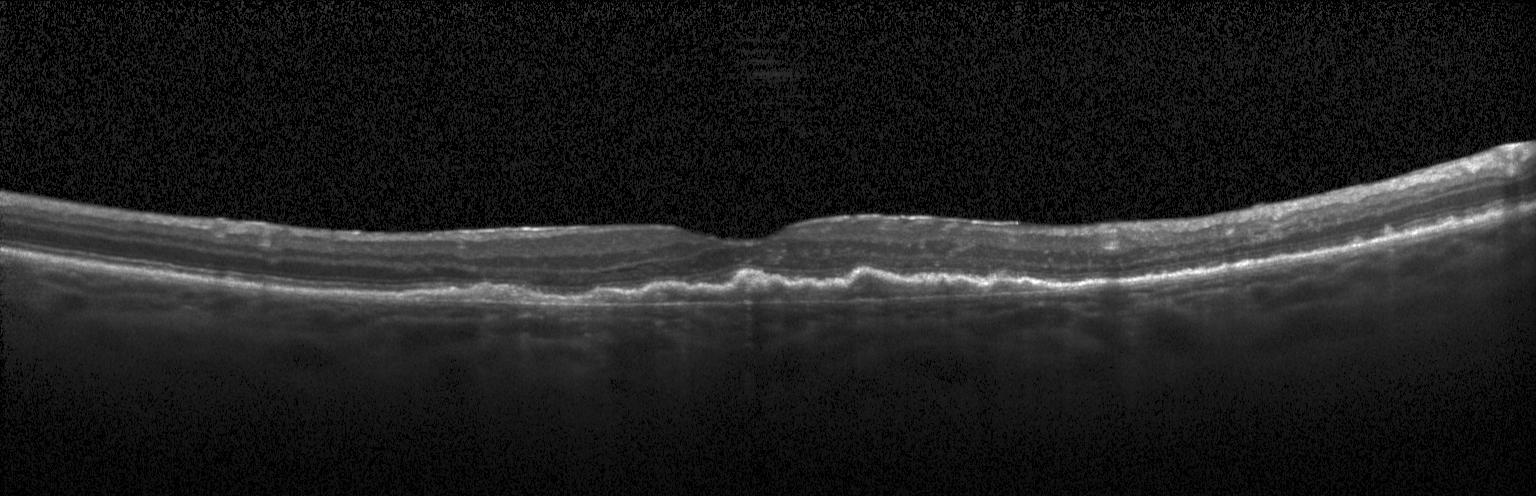
Optical coherence tomography scan.
OCT finding: a choroidal neovascular membrane.